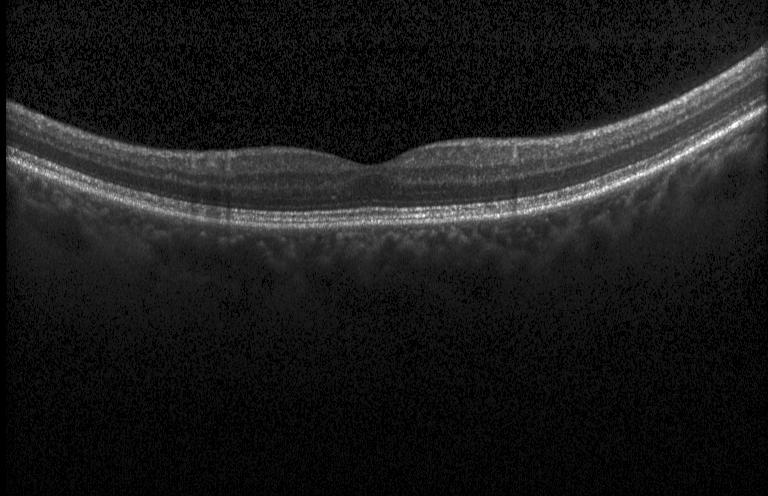
Through the macula. OCT line scan. Acquired on a Heidelberg Spectralis
Dx: neither choroidal neovascularization, diabetic macular edema, nor drusen.